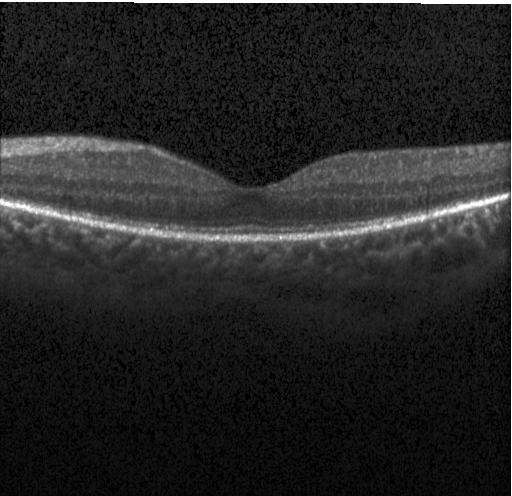
OCT scan showing neither choroidal neovascularization, diabetic macular edema, nor drusen.